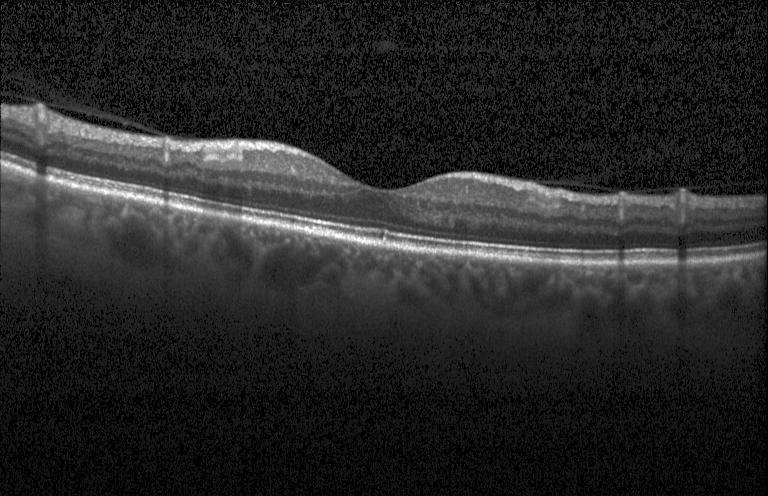
Acquired on a Heidelberg Spectralis, macular scan, retinal OCT cross-section — Diagnosis: no CNV, DME, or drusen.